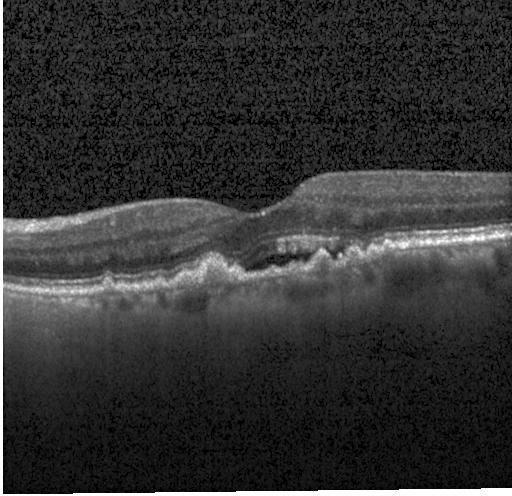
CNV.